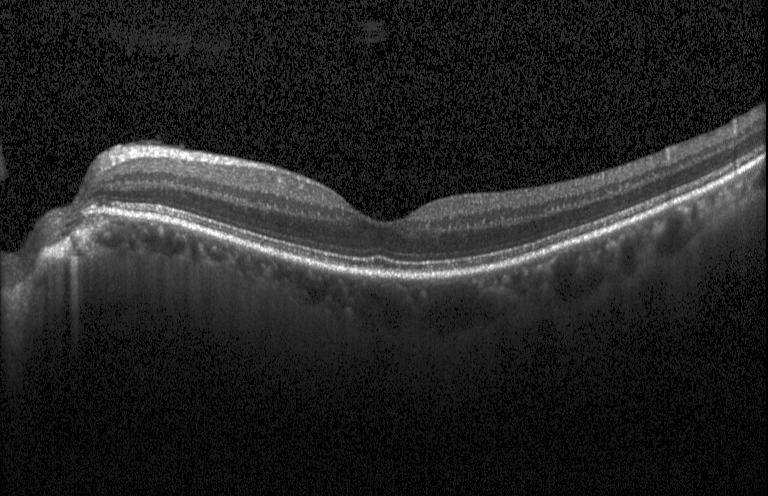

SD-OCT, horizontal scan through the fovea, Heidelberg Spectralis OCT system, retinal OCT B-scan
Dx: neither choroidal neovascularization, diabetic macular edema, nor drusen.